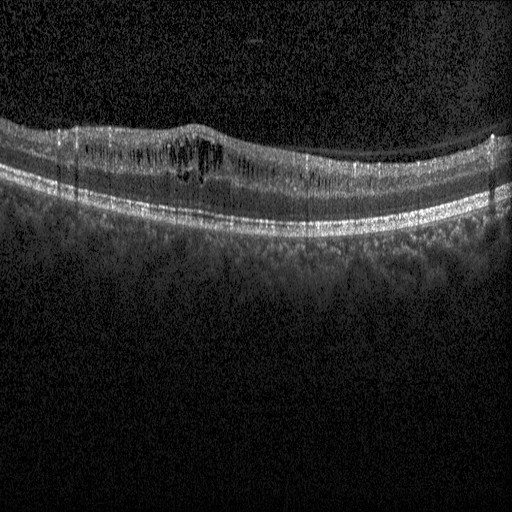
Retinal OCT cross-section. Finding: diabetic macular edema.